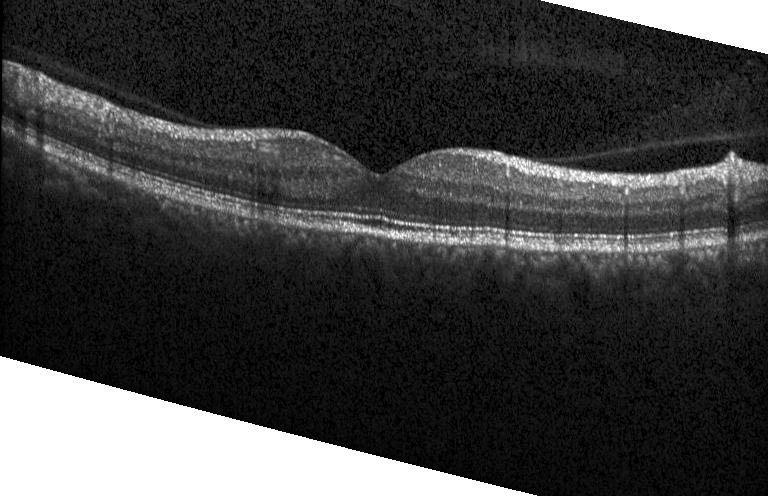

Spectral-domain OCT. Optical coherence tomography B-scan — Impression: neither choroidal neovascularization, diabetic macular edema, nor drusen.